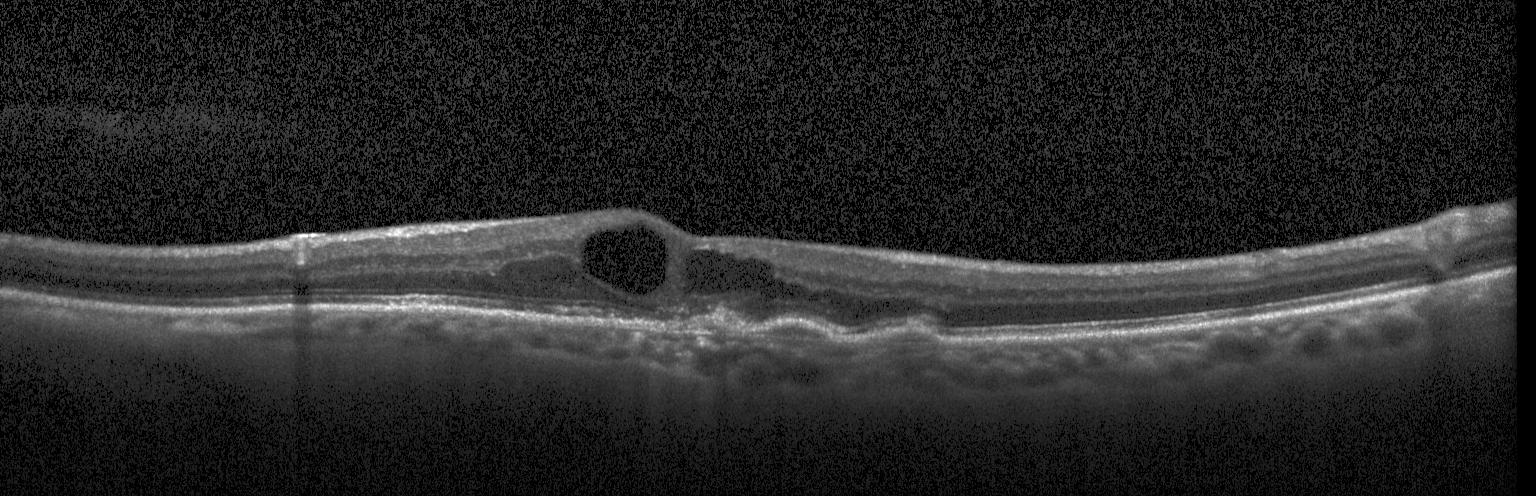
Optical coherence tomography scan · through the macula.
Assessment: choroidal neovascularization.